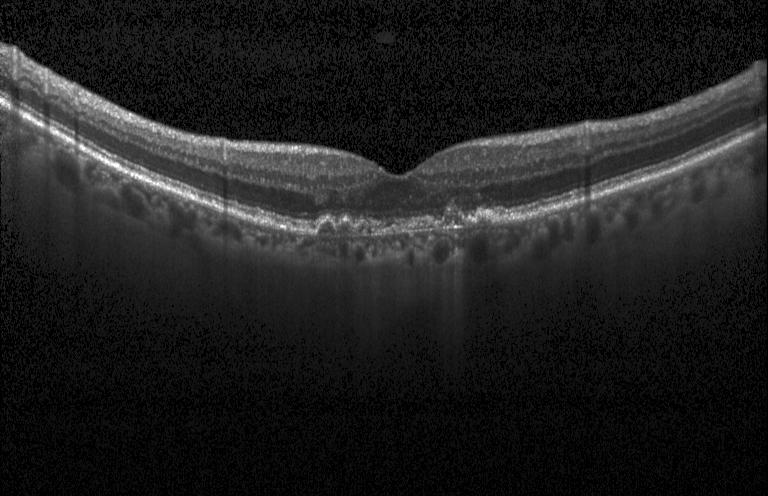 Centered on the fovea · spectral-domain OCT · optical coherence tomography B-scan. The scan shows drusen.